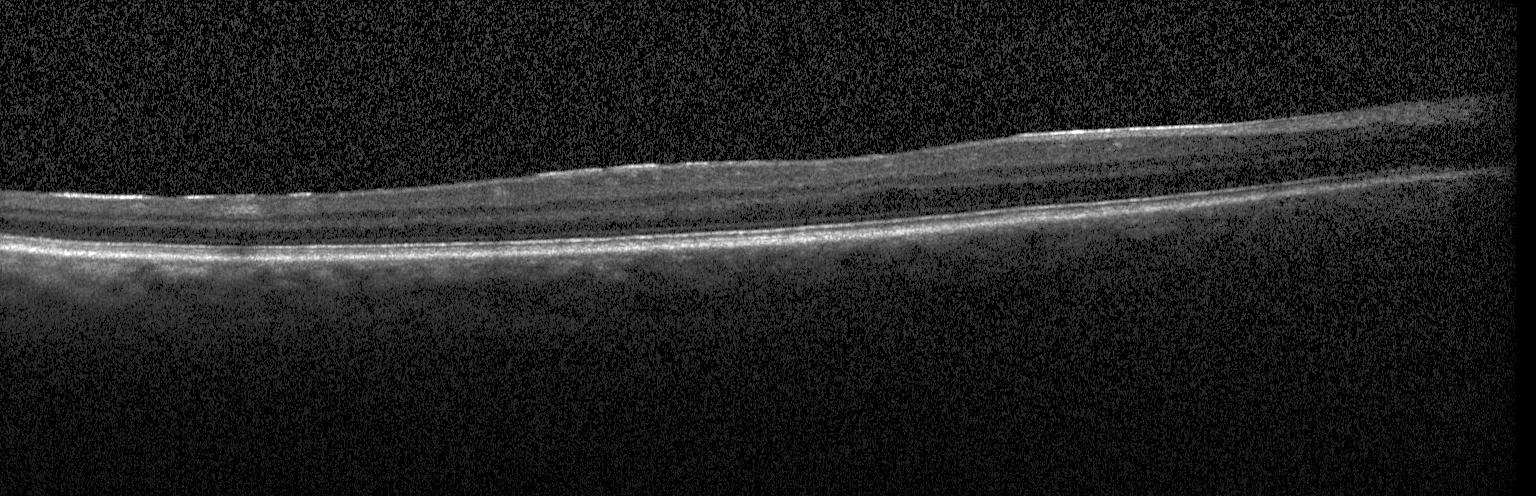

Centered on the fovea. Acquired on a Heidelberg Spectralis. OCT B-scan.
Impression: no evidence of choroidal neovascularization, diabetic macular edema, or drusen.